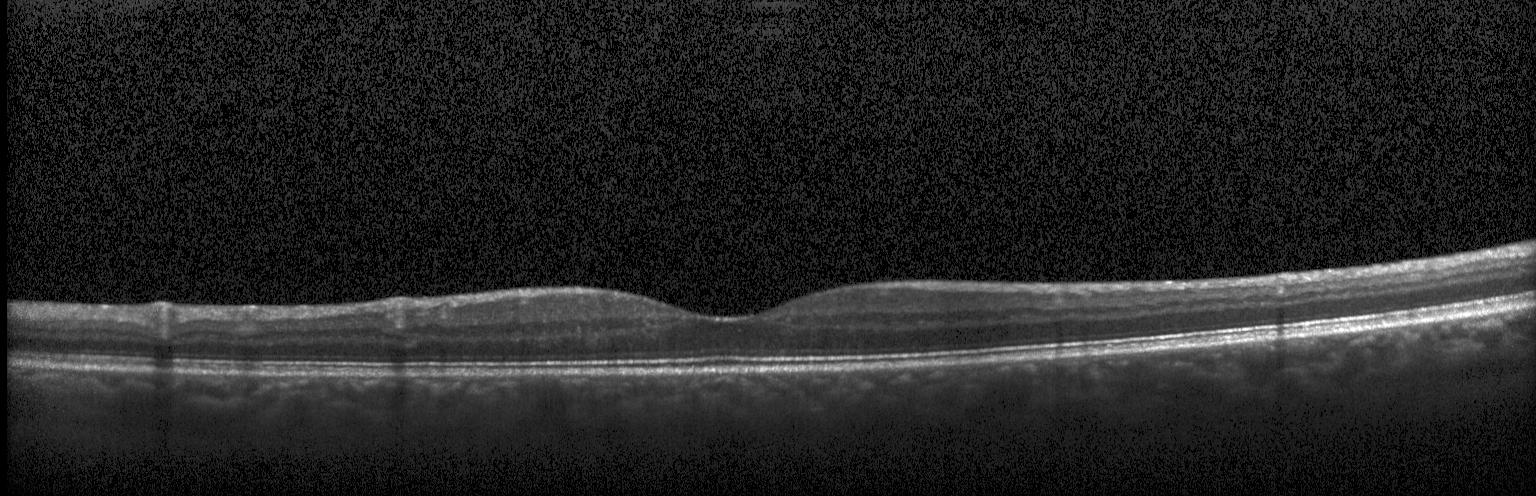 OCT line scan; horizontal scan through the fovea. This B-scan demonstrates neither choroidal neovascularization, diabetic macular edema, nor drusen.